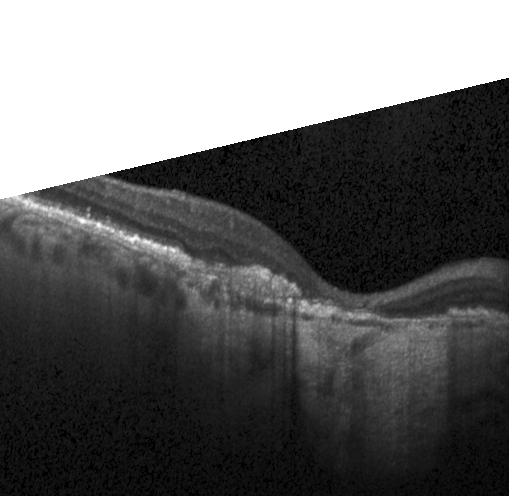
A choroidal neovascular membrane.